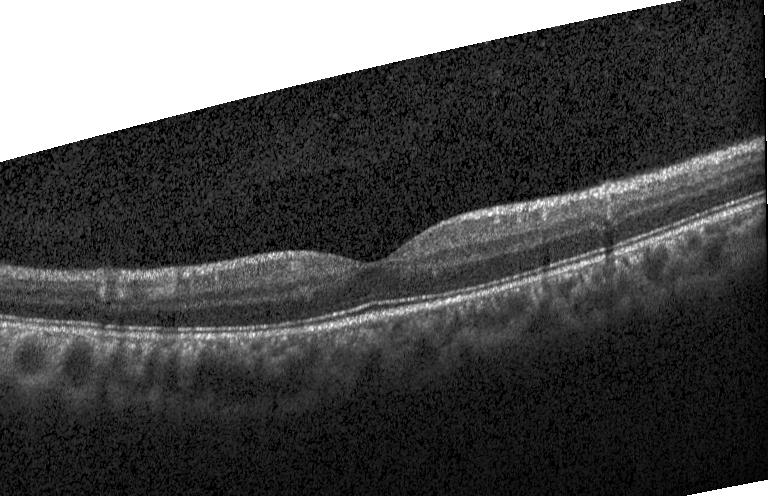 Instrument: Heidelberg Spectralis, optical coherence tomography scan.
This B-scan demonstrates no CNV, no DME, and no drusen.